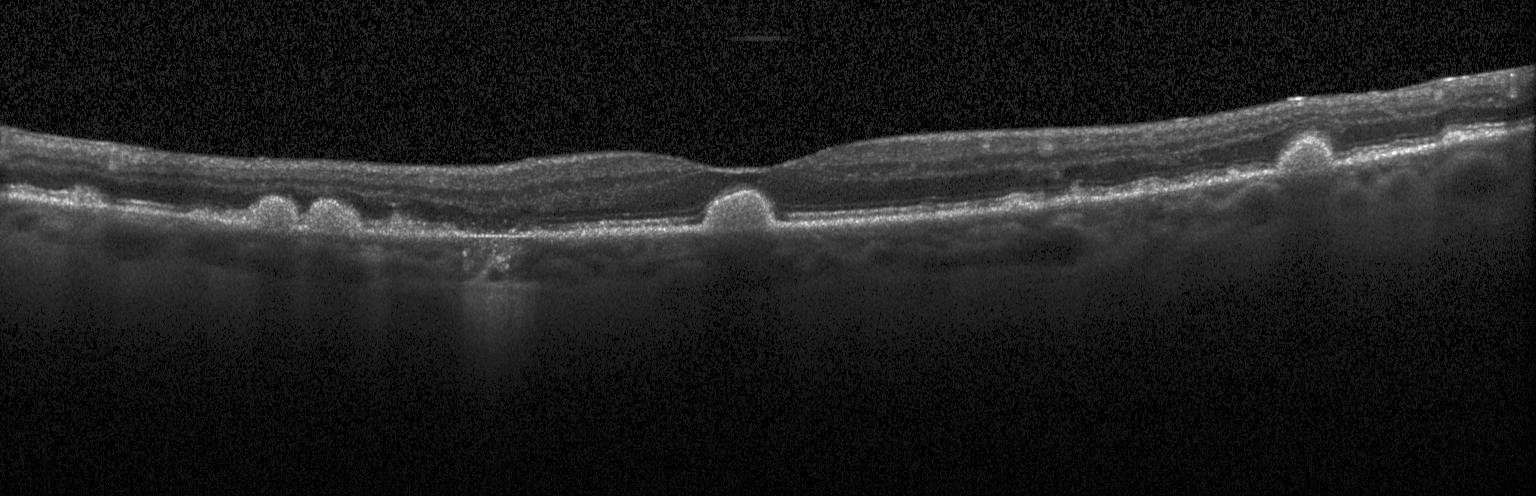

OCT B-scan showing sub-RPE drusenoid deposits.